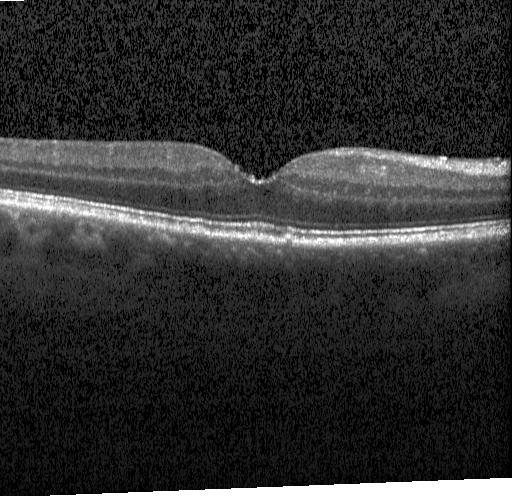 Spectral-domain OCT B-scan: sub-RPE drusenoid deposits.